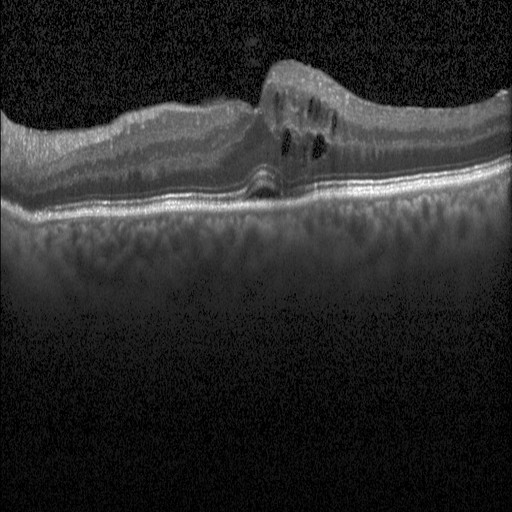
Impression: diabetic macular edema (DME).